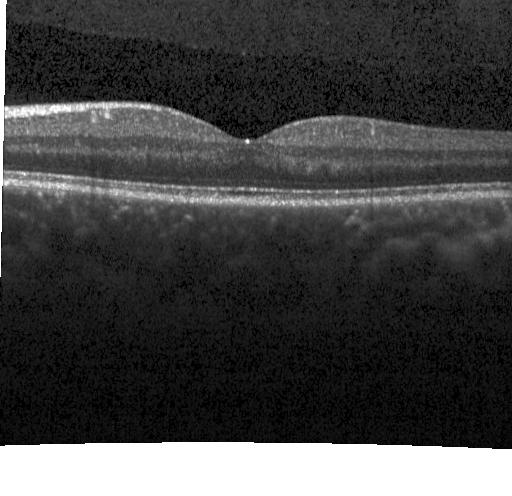 Retinal OCT cross-section showing no evidence of choroidal neovascularization, diabetic macular edema, or drusen.